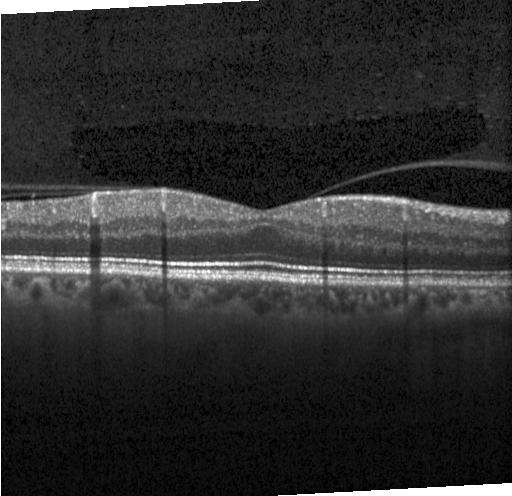 Spectral-domain optical coherence tomography. Through the macula. OCT B-scan. Instrument: Heidelberg Spectralis. Impression: no choroidal neovascularization, no diabetic macular edema, and no drusen.